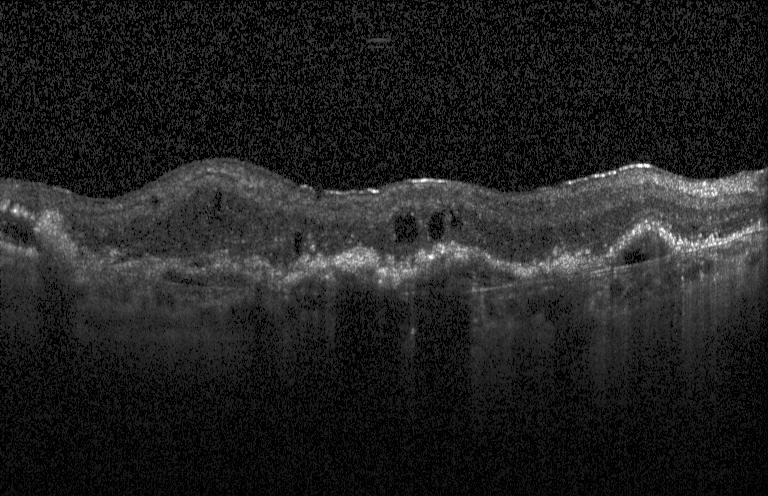 Spectral-domain OCT B-scan: CNV.